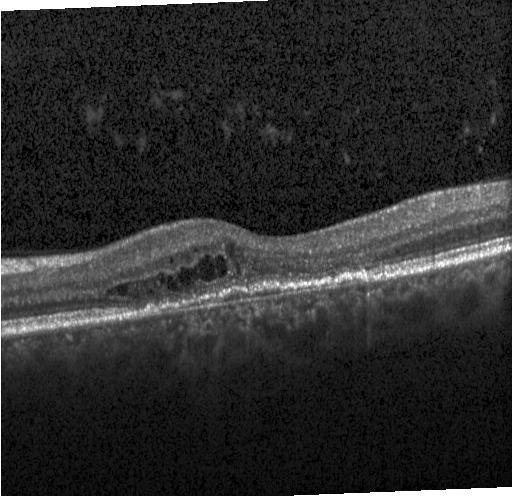 Impression: CNV.